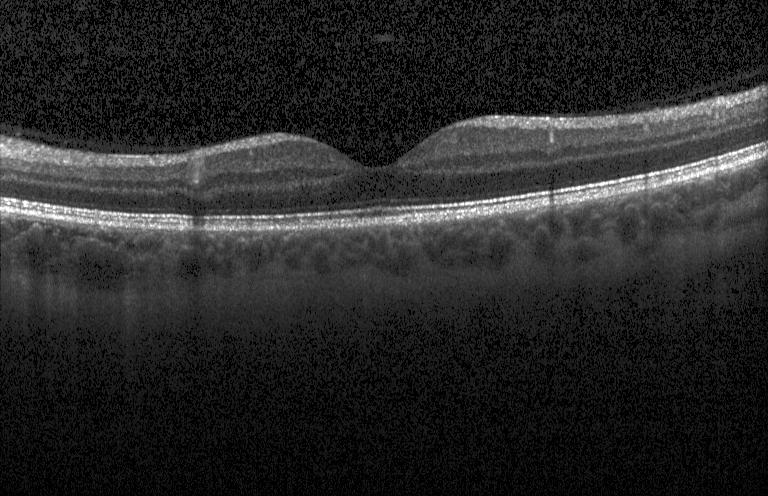 OCT line scan. Spectral-domain optical coherence tomography
Diagnosis: no choroidal neovascularization, diabetic macular edema, or drusen.